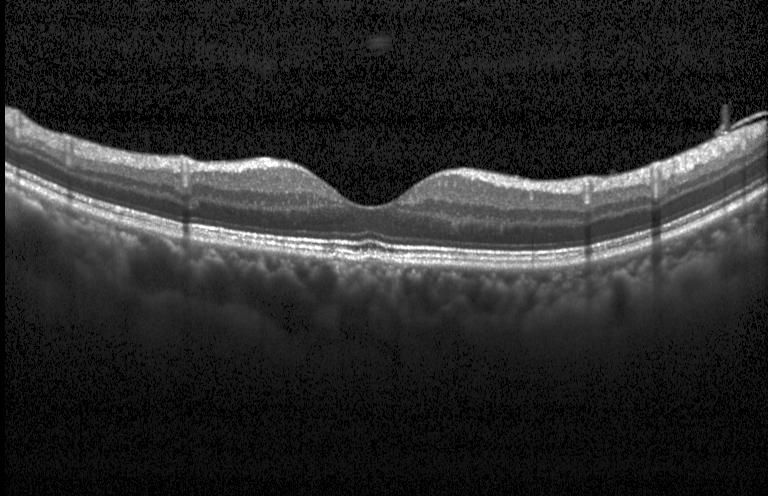

Retinal OCT B-scan. No CNV, no DME, and no drusen.